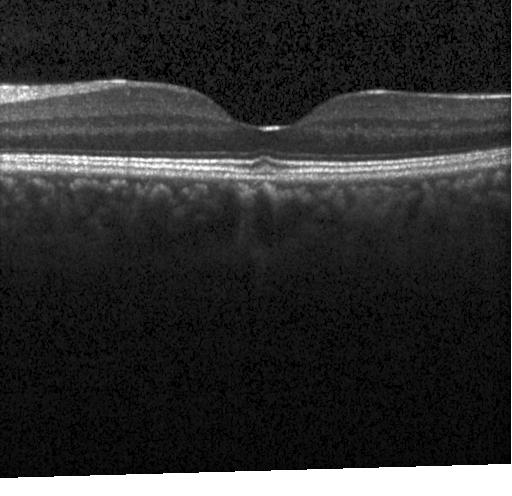
OCT scan showing no choroidal neovascularization, no diabetic macular edema, and no drusen.